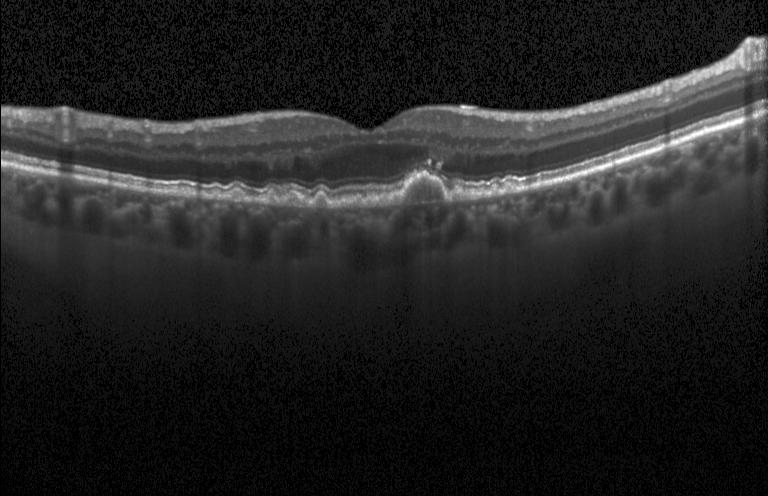 Retinal OCT cross-section showing a choroidal neovascular membrane.